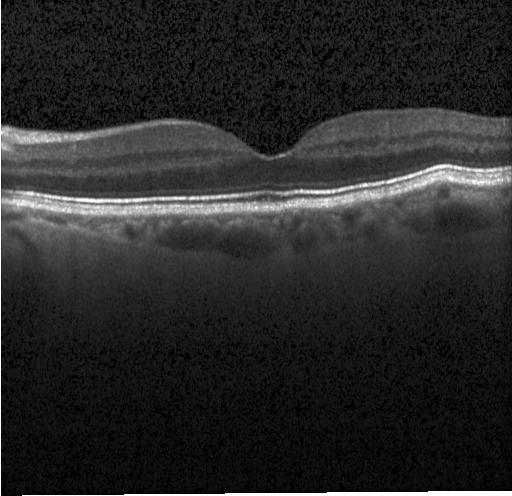

Optical coherence tomography scan.
Assessment: neither choroidal neovascularization, diabetic macular edema, nor drusen.